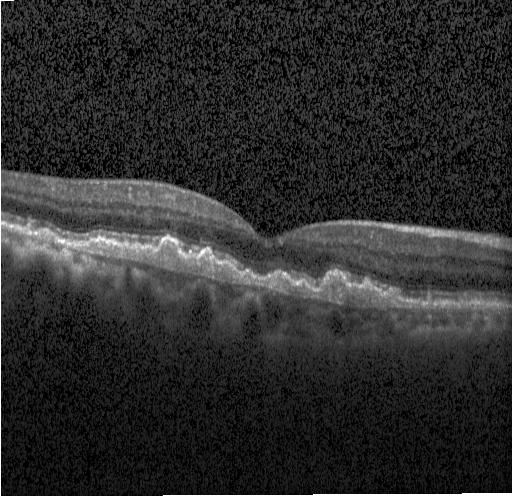
Diagnosis: CNV.